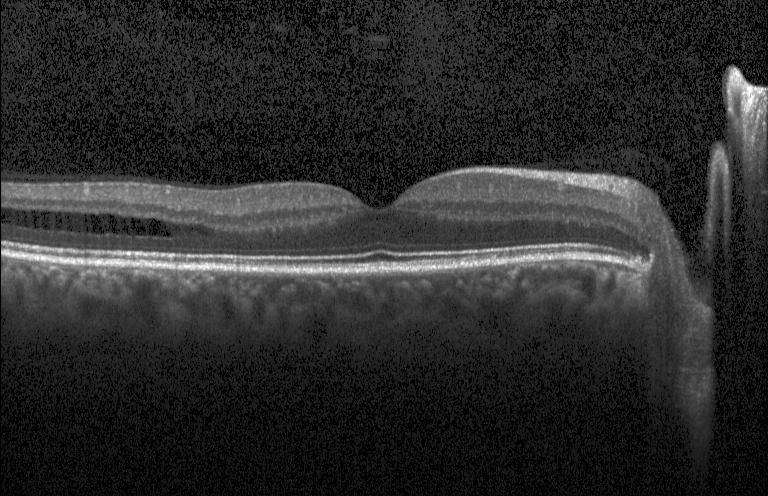
Retinal OCT B-scan, instrument: Heidelberg Spectralis, SD-OCT — Impression: no evidence of CNV, DME, or drusen.